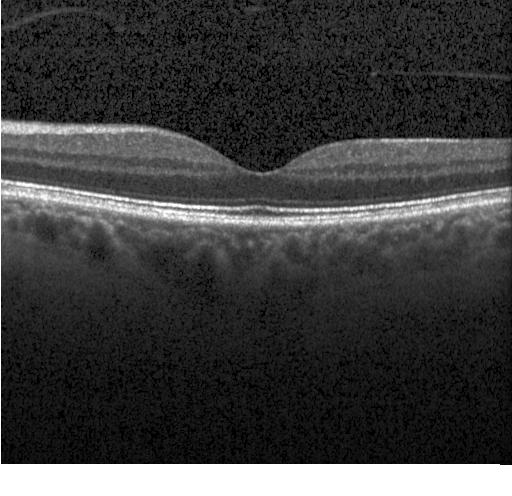 OCT B-scan showing no evidence of CNV, DME, or drusen.